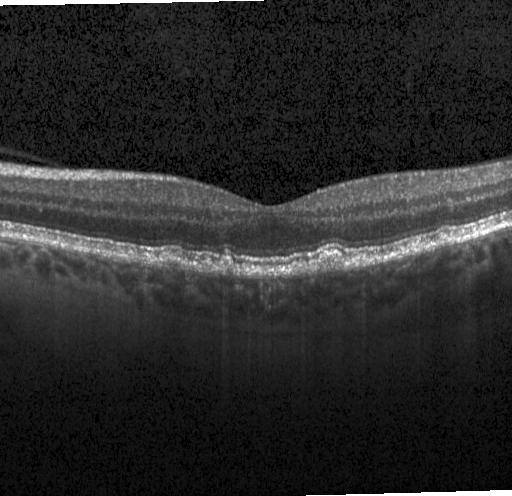
SD-OCT. Horizontal scan through the fovea. Heidelberg Spectralis. Optical coherence tomography B-scan.
OCT finding: multiple drusen.